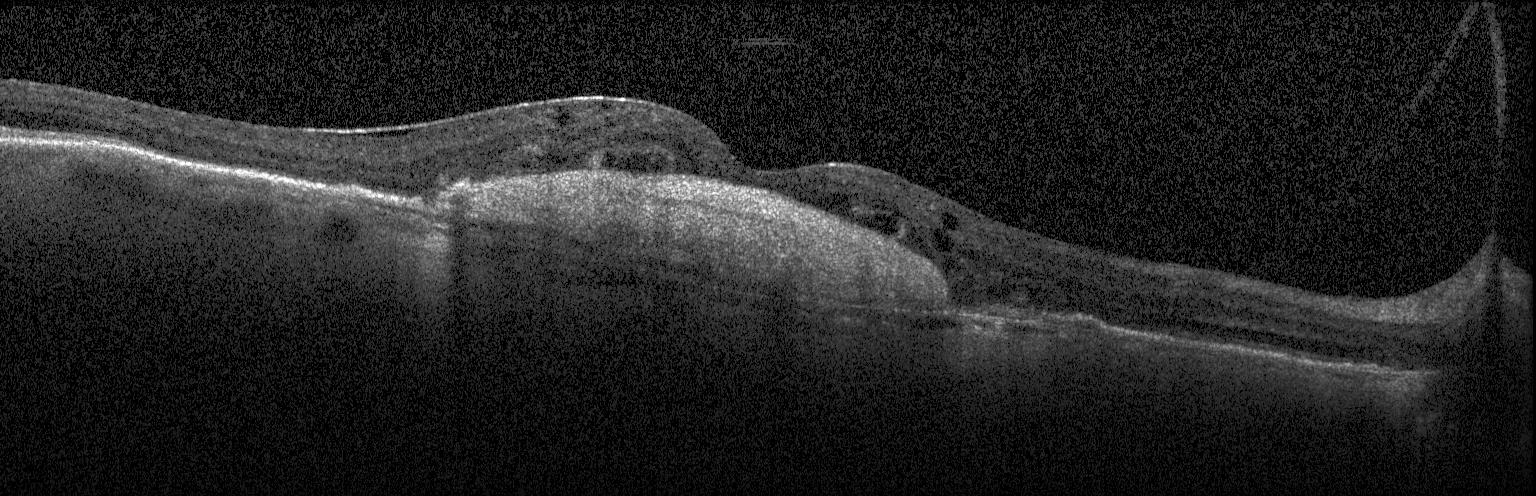 Diagnosis: choroidal neovascularization.